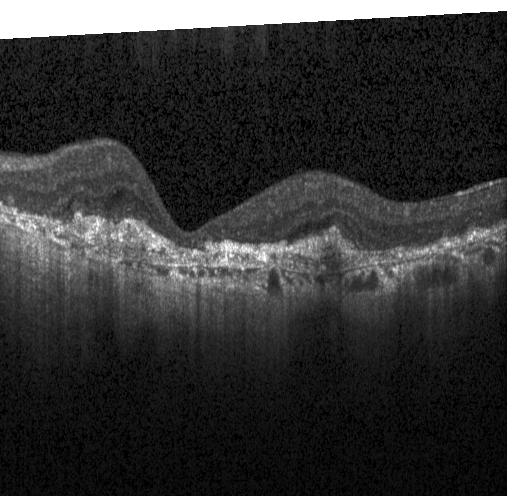

Assessment: choroidal neovascularization.